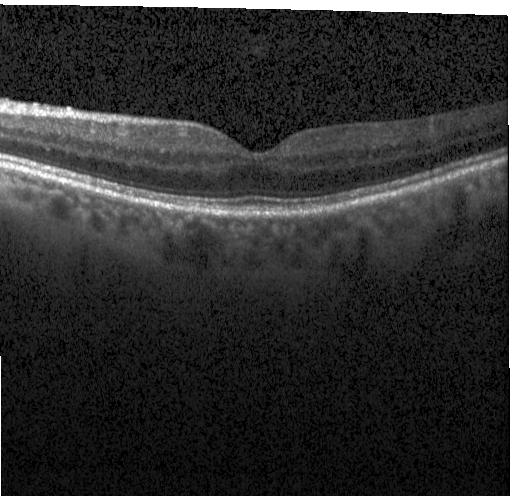 OCT line scan. Heidelberg Spectralis OCT system — Assessment: no evidence of choroidal neovascularization, diabetic macular edema, or drusen.